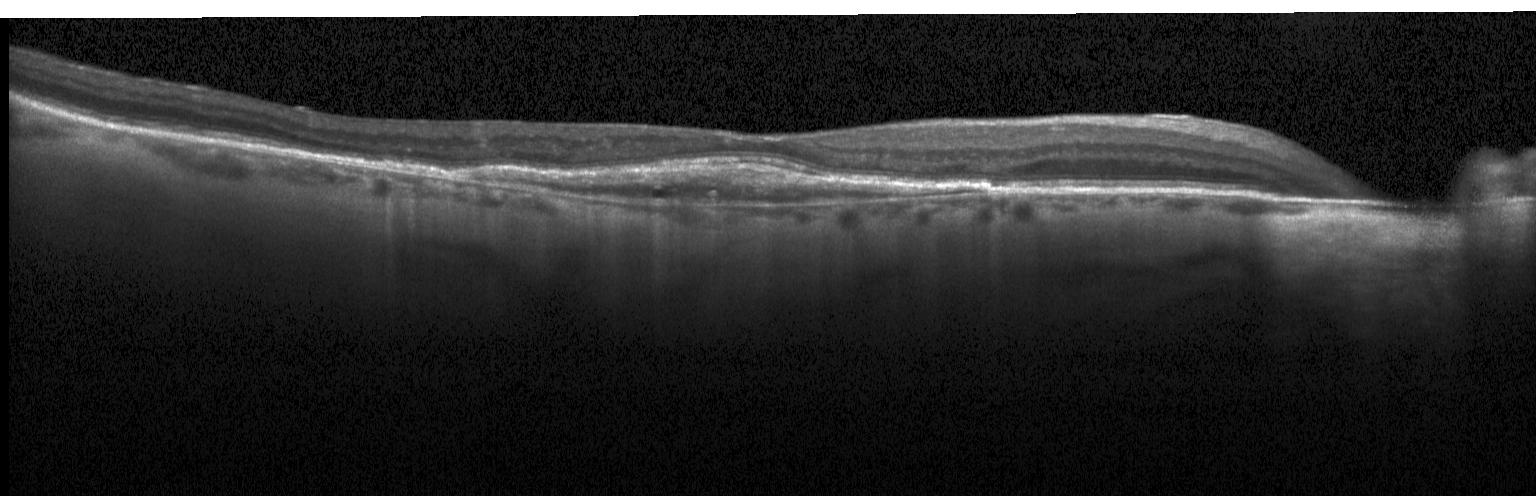 OCT scan showing choroidal neovascularization.